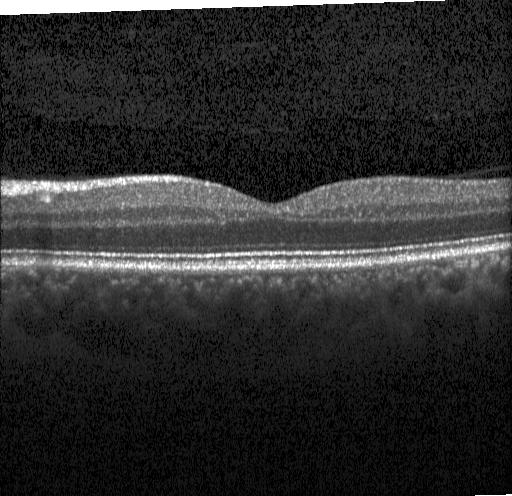
Finding: no choroidal neovascularization, diabetic macular edema, or drusen.